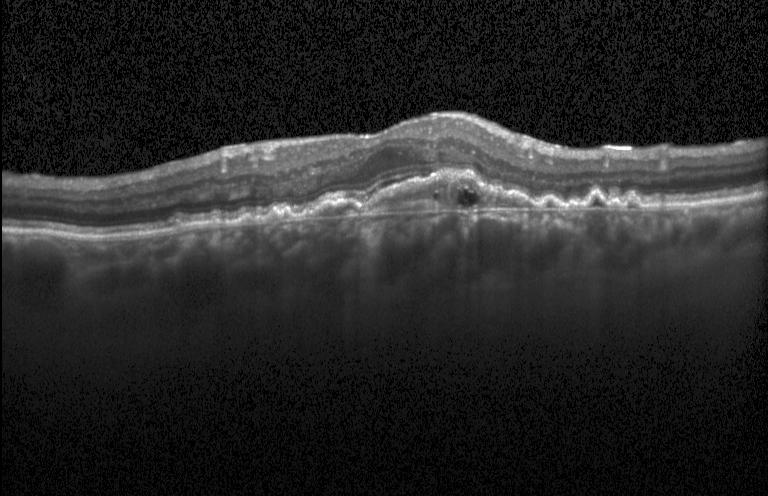
Finding: a choroidal neovascular membrane.